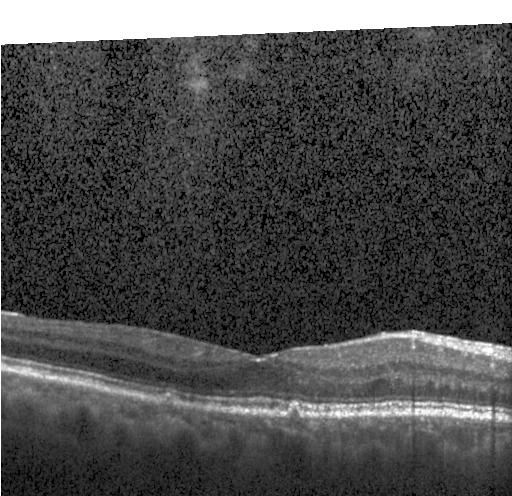 Retinal OCT B-scan · Heidelberg Spectralis OCT system · through the macula.
Diagnosis: sub-RPE drusenoid deposits.